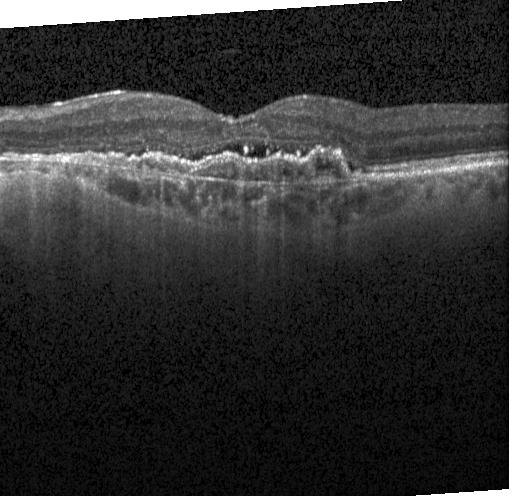

Fovea-centered · OCT line scan · SD-OCT · acquired on a Heidelberg Spectralis.
OCT finding: a choroidal neovascular membrane.